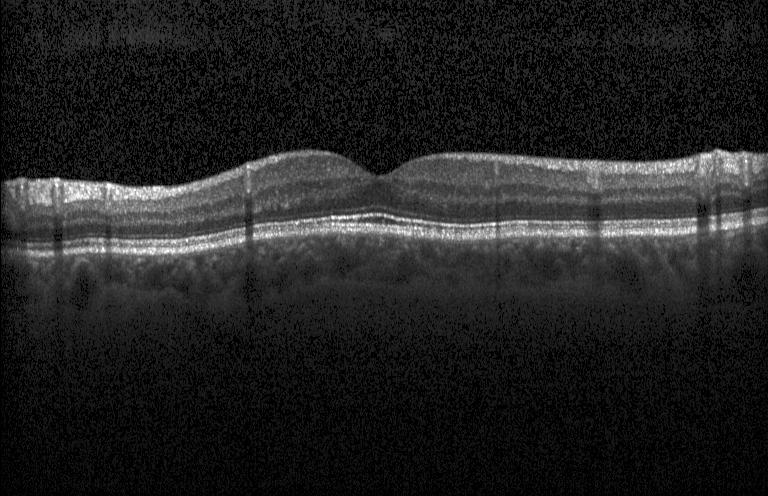

Optical coherence tomography scan. Fovea-centered — Impression: no choroidal neovascularization, diabetic macular edema, or drusen.